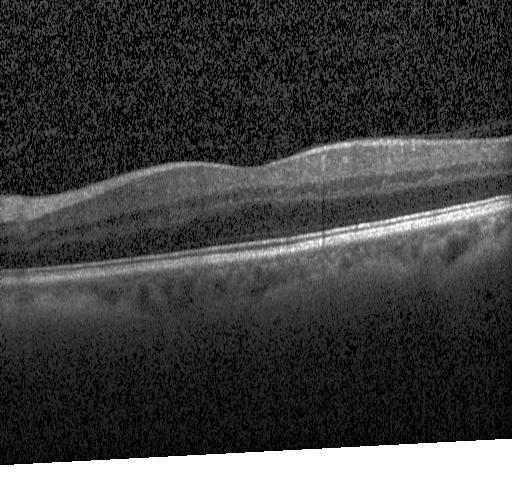 No choroidal neovascularization, no diabetic macular edema, and no drusen.